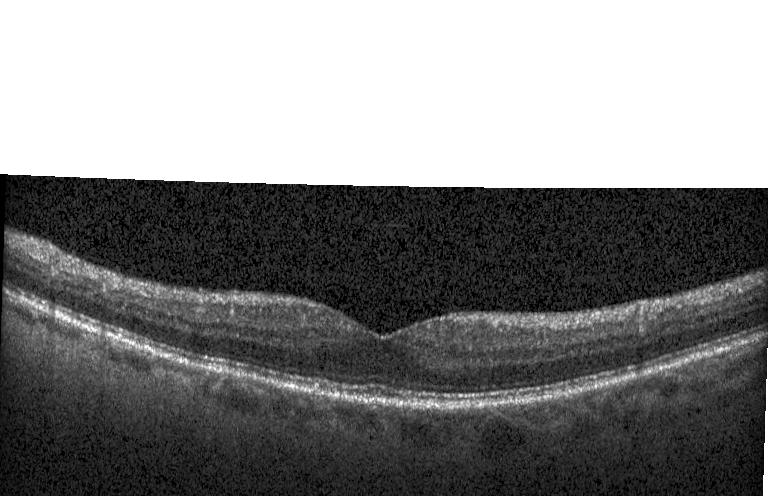
Retinal OCT cross-section showing neither CNV, DME, nor drusen.